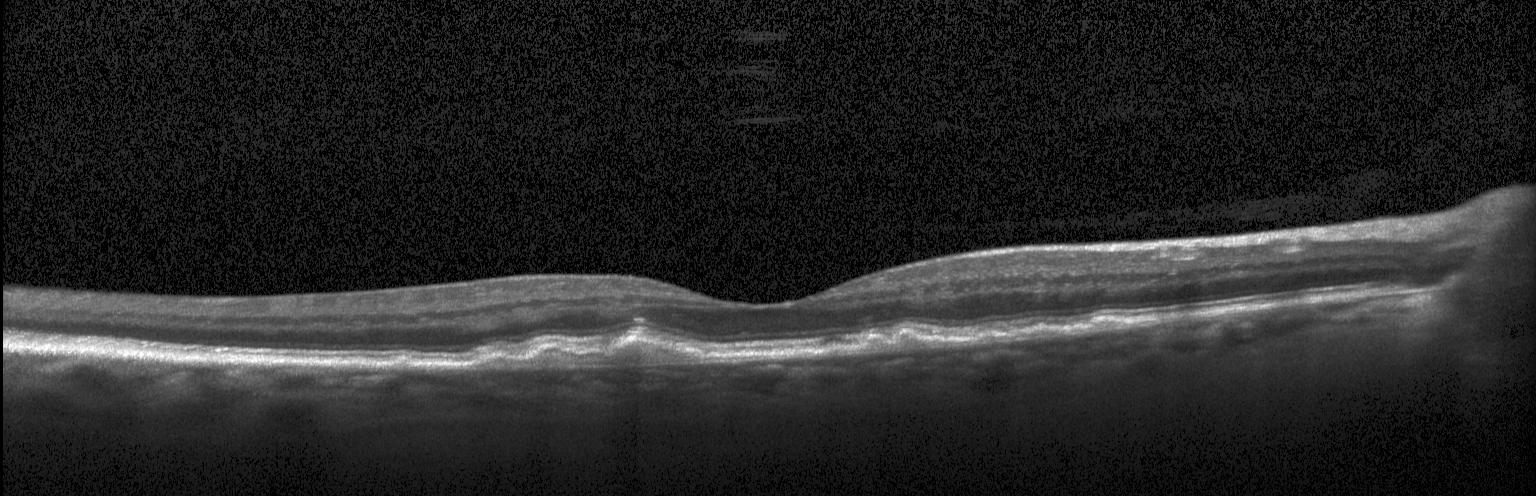

OCT line scan; through the macula; SD-OCT; Heidelberg Spectralis OCT system. Impression: multiple drusen.